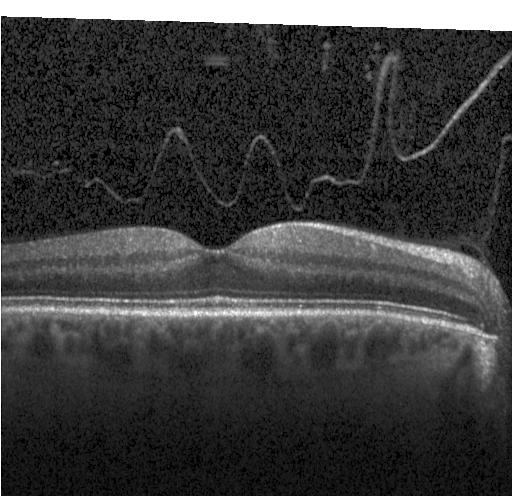
Through the macula · optical coherence tomography B-scan · Heidelberg Spectralis OCT system — Impression: no evidence of choroidal neovascularization, diabetic macular edema, or drusen.